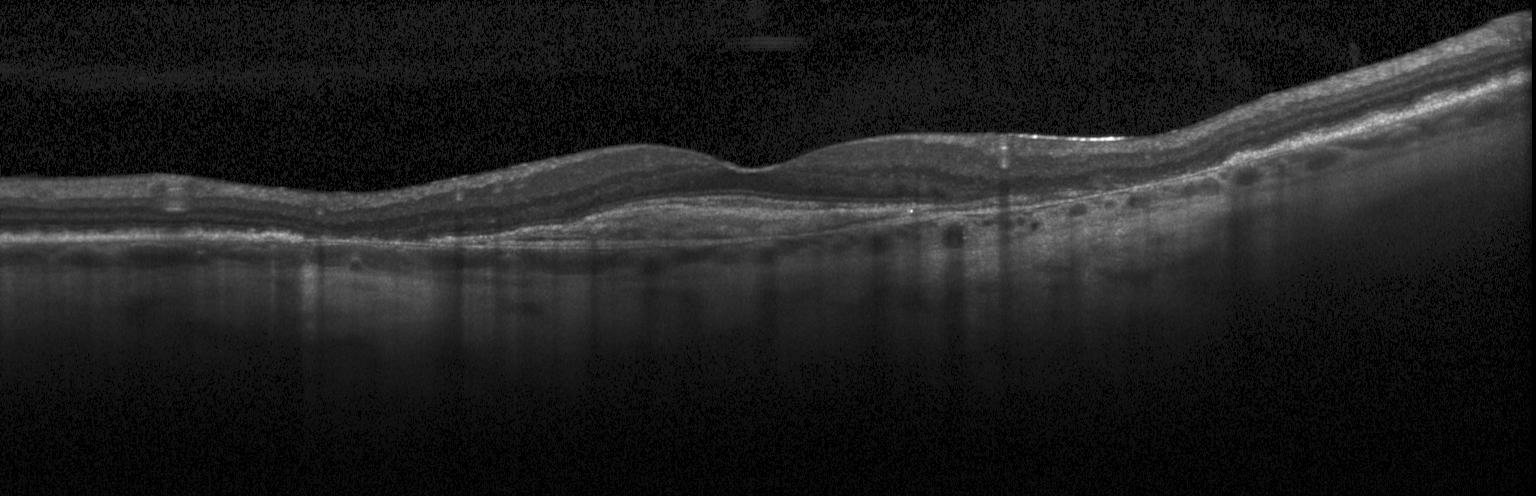 Impression: CNV.